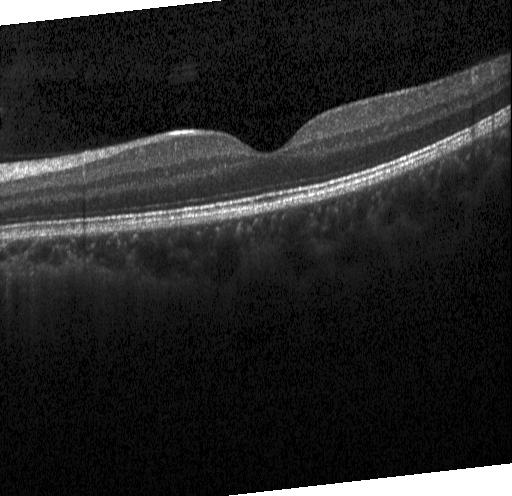 Macular OCT: no CNV, no DME, and no drusen.